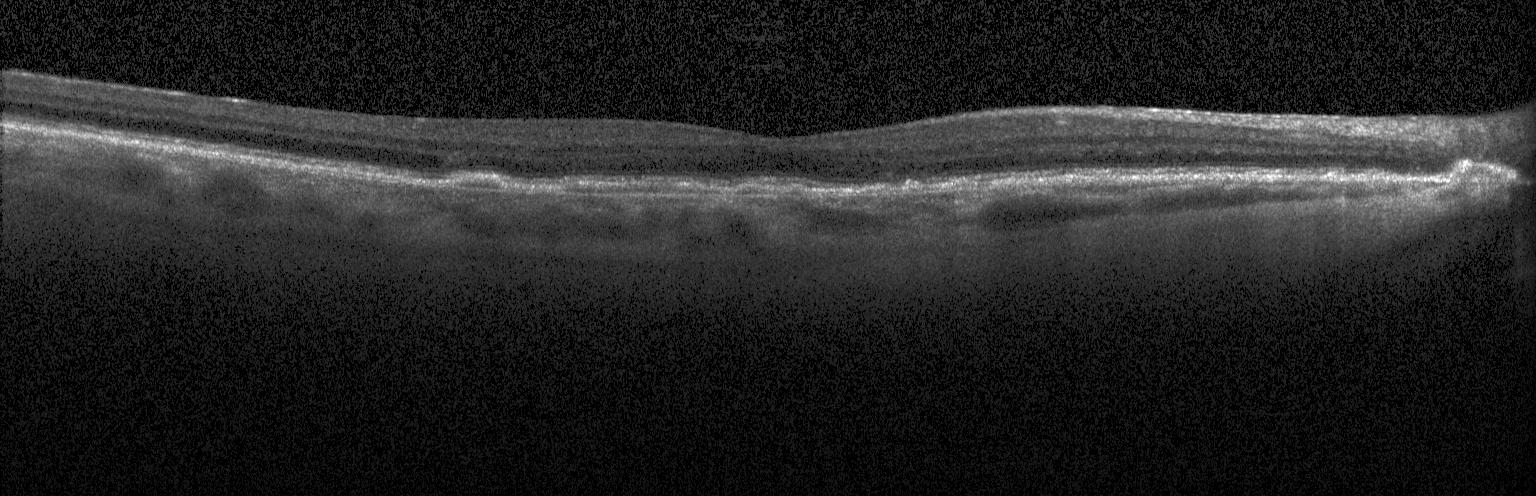

Finding: a choroidal neovascular membrane.